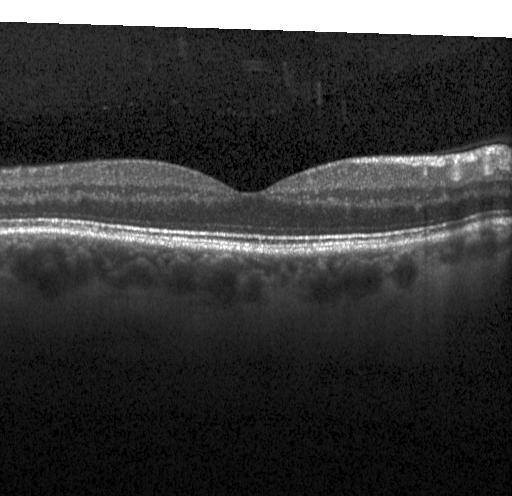

Retinal OCT B-scan — Dx: no choroidal neovascularization, no diabetic macular edema, and no drusen.